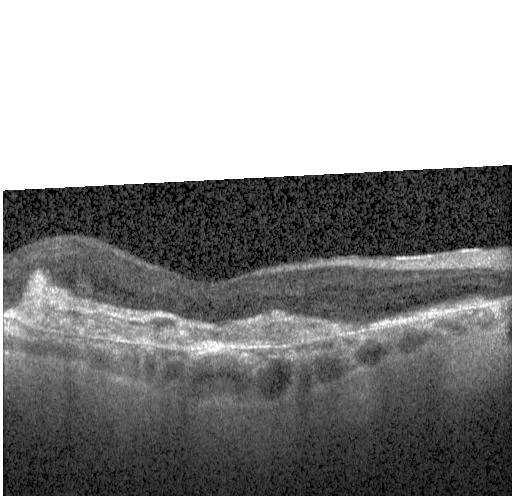

Optical coherence tomography B-scan.
Finding: choroidal neovascularization (CNV).